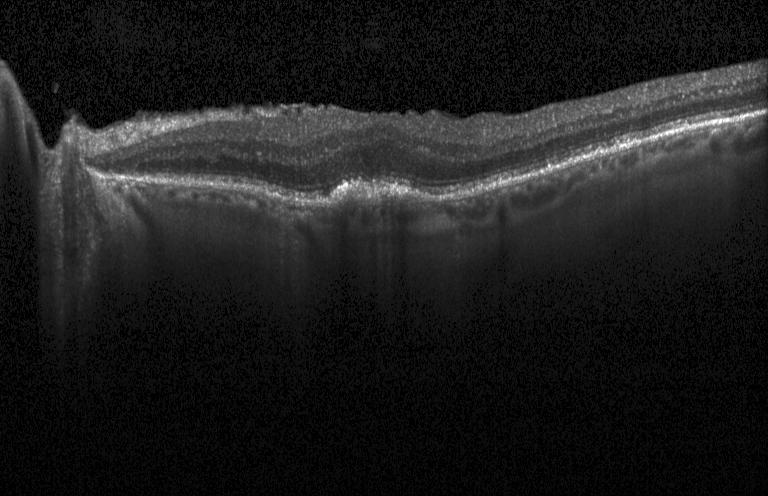
Macular OCT demonstrating a choroidal neovascular membrane.